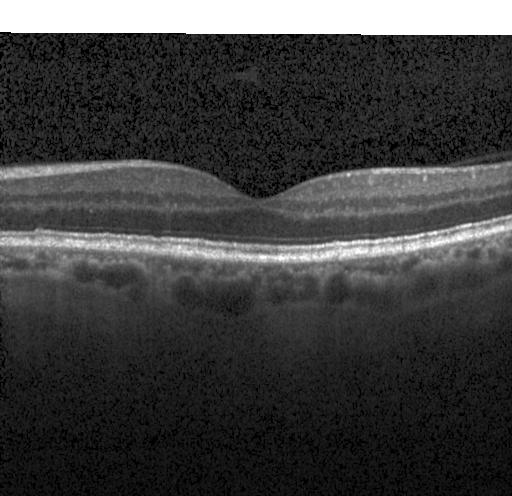 OCT scan showing neither CNV, DME, nor drusen.